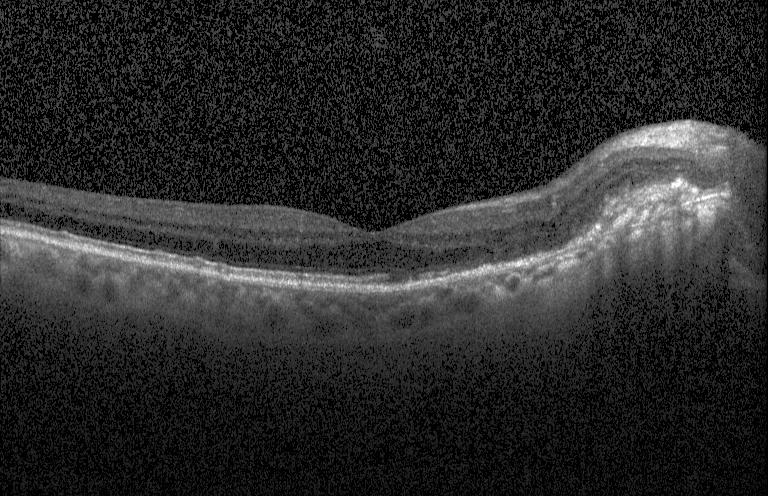

The scan shows choroidal neovascularization.